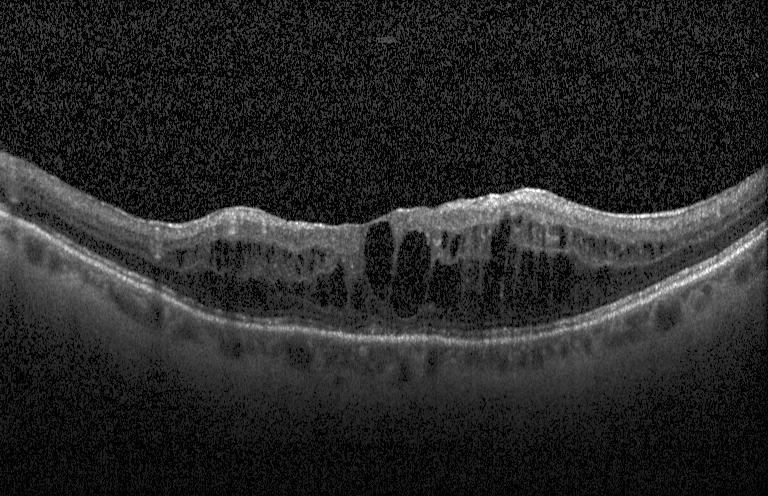
Fovea-centered, retinal OCT B-scan, SD-OCT — Assessment: DME.